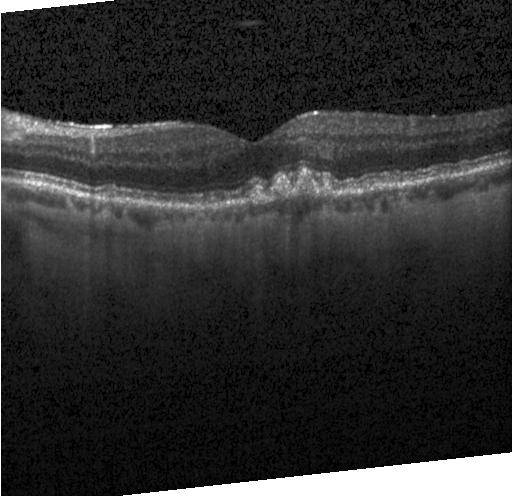
Impression: drusen.